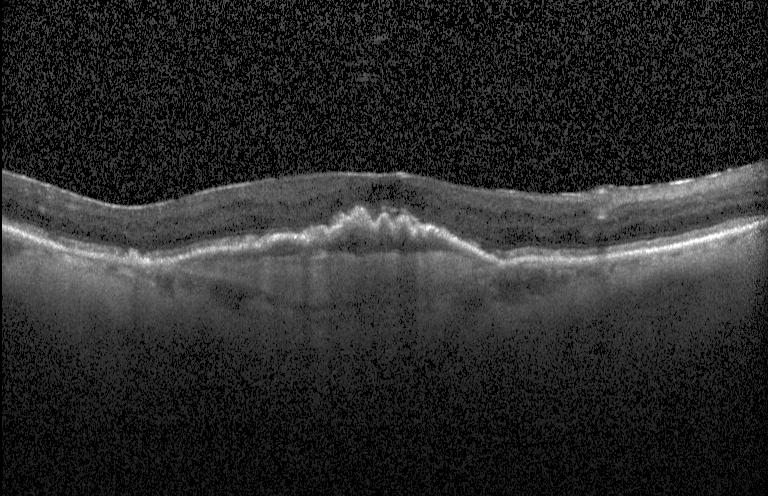 OCT scan showing a choroidal neovascular membrane.